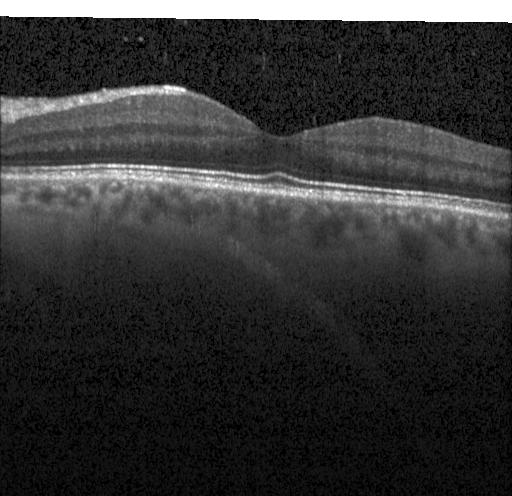 Finding: neither choroidal neovascularization, diabetic macular edema, nor drusen.